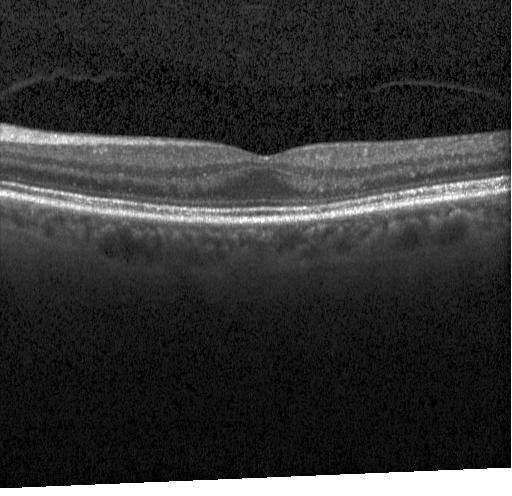 OCT scan showing neither CNV, DME, nor drusen.